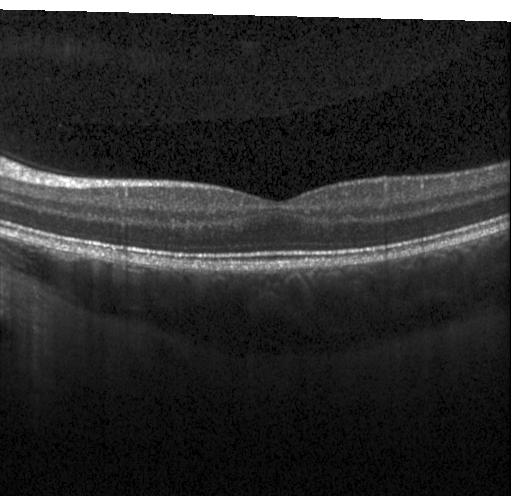

Retinal OCT cross-section showing neither CNV, DME, nor drusen.